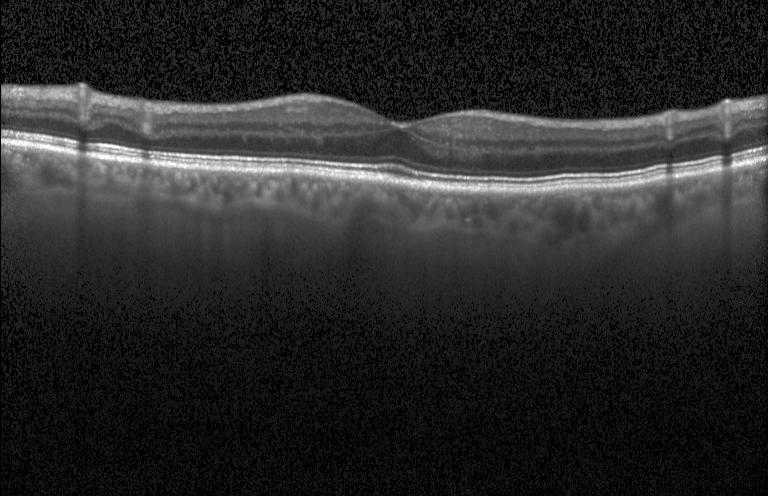 Acquired on a Heidelberg Spectralis · horizontal scan through the fovea · optical coherence tomography B-scan · spectral-domain OCT.
Neither choroidal neovascularization, diabetic macular edema, nor drusen.